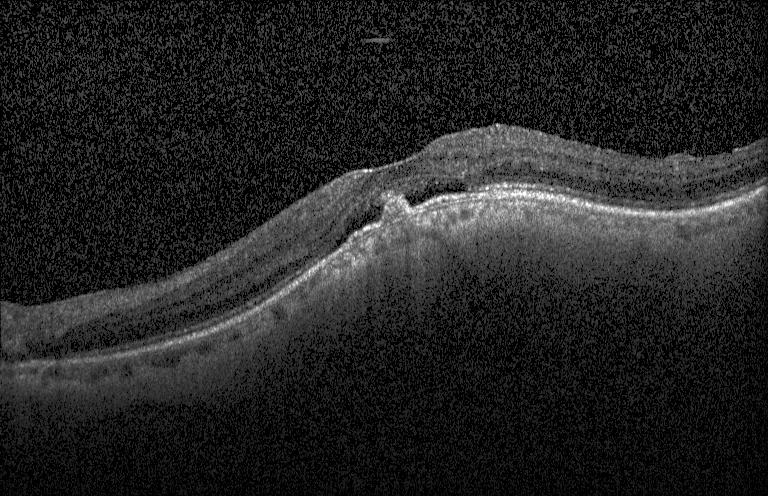 Assessment: choroidal neovascularization.